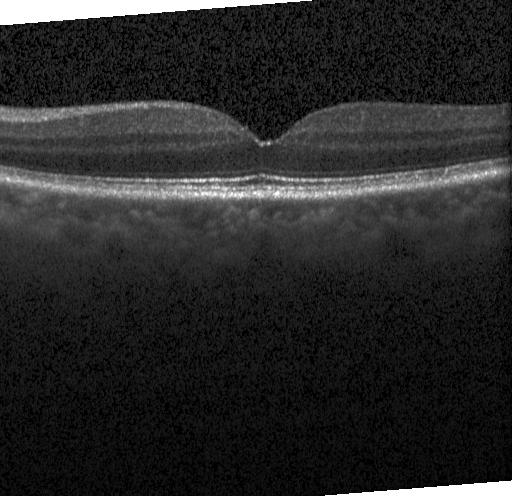

Spectral-domain OCT B-scan: no CNV, no DME, and no drusen.